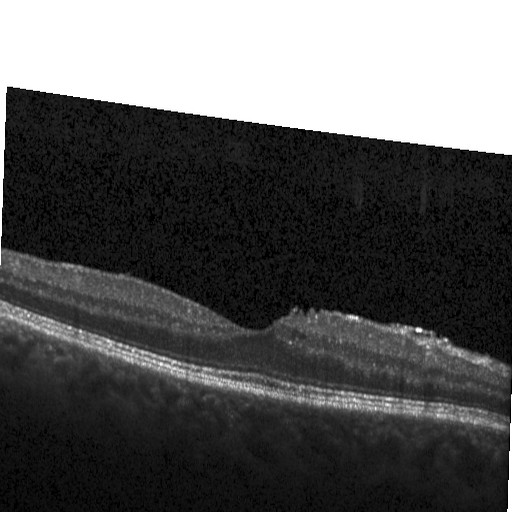 OCT B-scan. Through the macula. Spectral-domain OCT. Impression: diabetic macular edema.